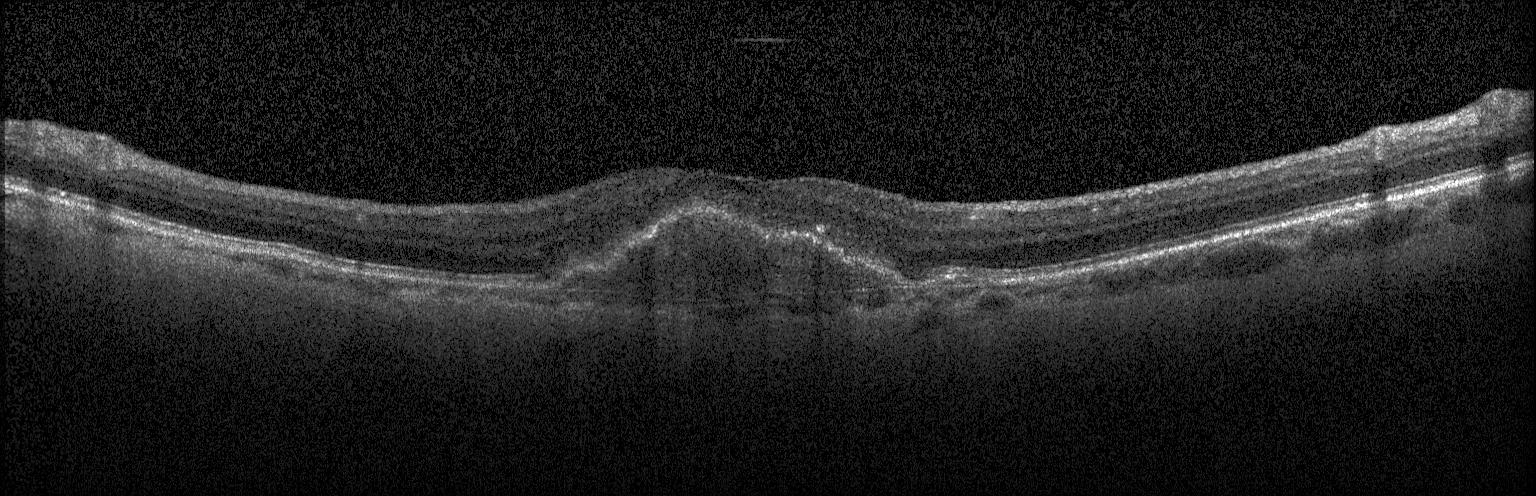 OCT finding: CNV.